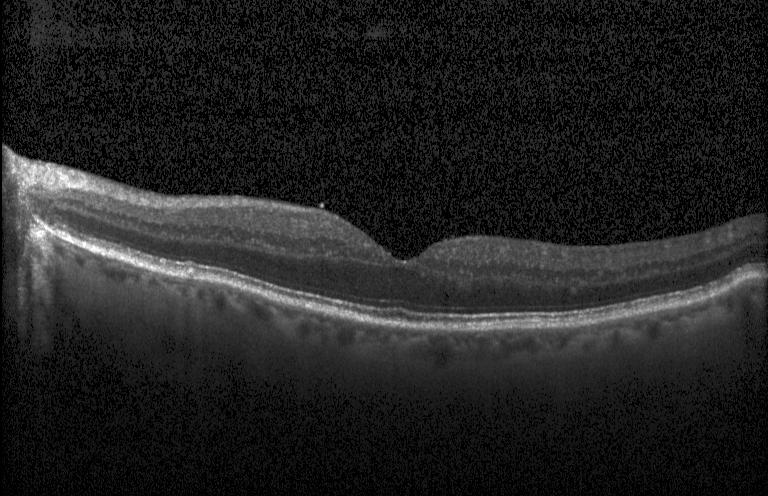
This B-scan demonstrates no choroidal neovascularization, diabetic macular edema, or drusen.